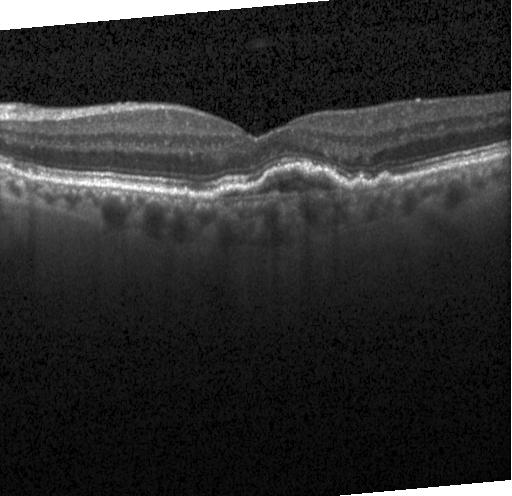
Spectral-domain OCT B-scan: a choroidal neovascular membrane.